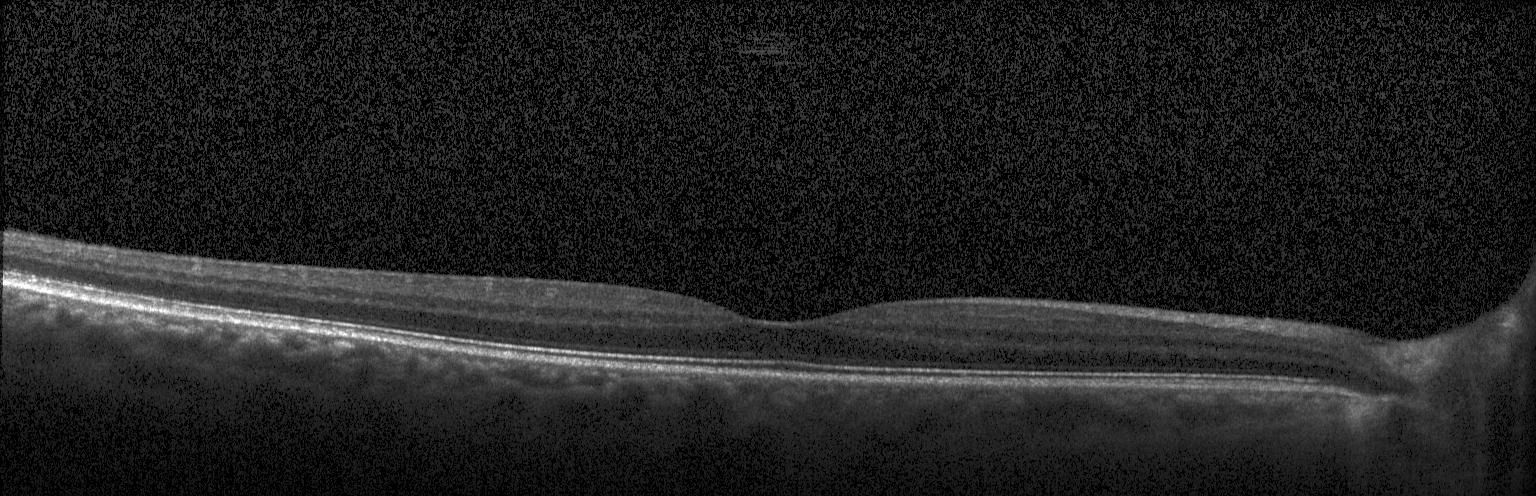
Heidelberg Spectralis OCT system · optical coherence tomography scan — Dx: no evidence of choroidal neovascularization, diabetic macular edema, or drusen.